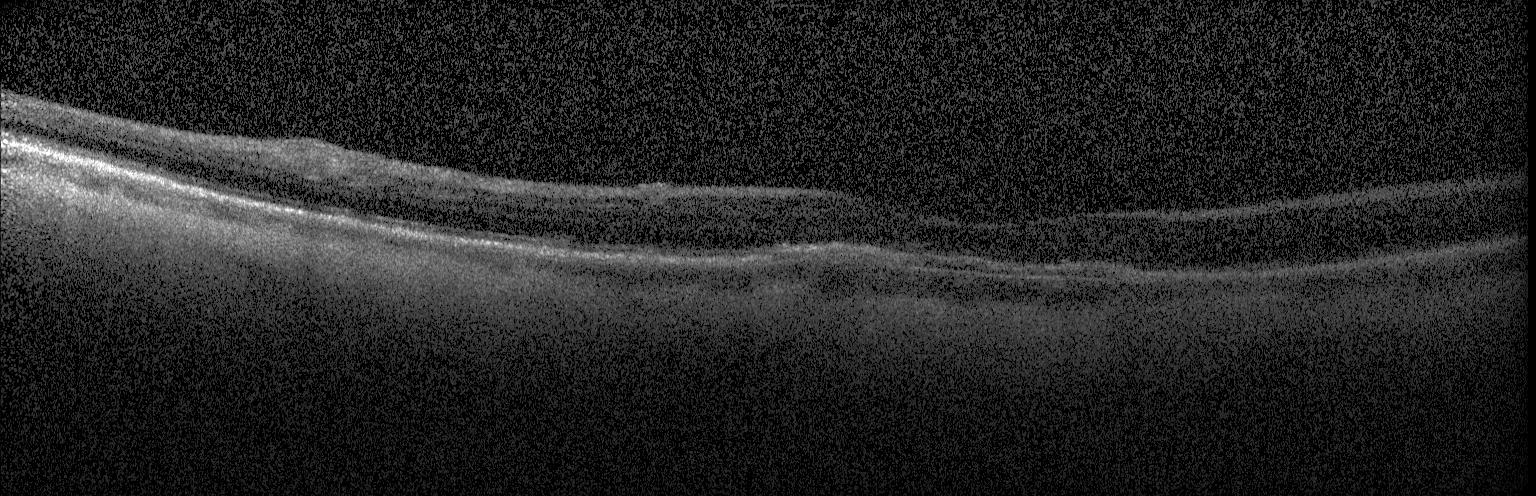

Retinal OCT cross-section showing choroidal neovascularization (CNV).